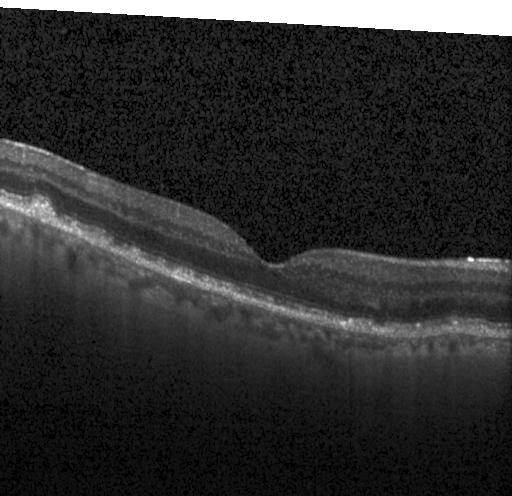 Fovea-centered; OCT B-scan.
OCT finding: drusen.